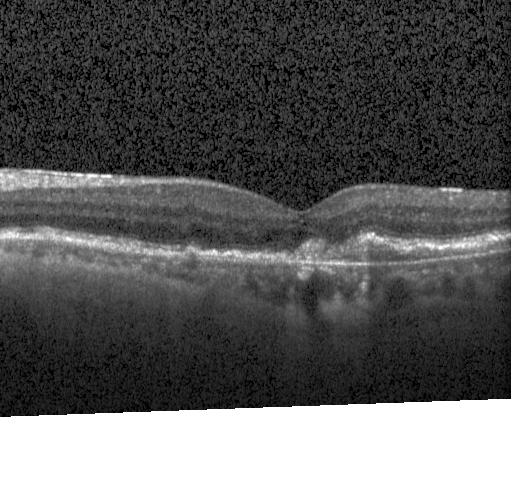

SD-OCT. OCT B-scan. Fovea-centered. Heidelberg Spectralis — OCT finding: CNV.